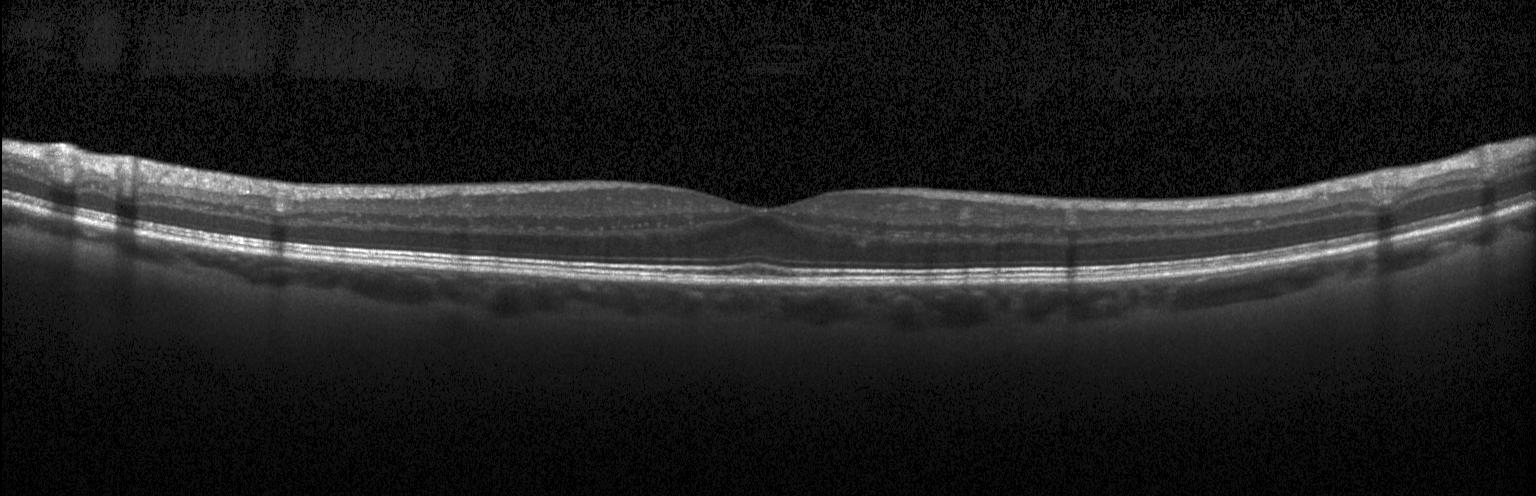
OCT line scan. No choroidal neovascularization, no diabetic macular edema, and no drusen.